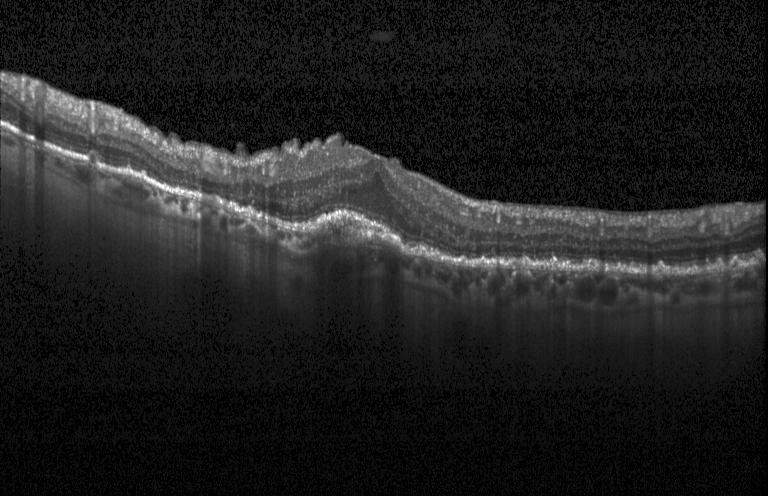 OCT B-scan.
This B-scan demonstrates choroidal neovascularization.